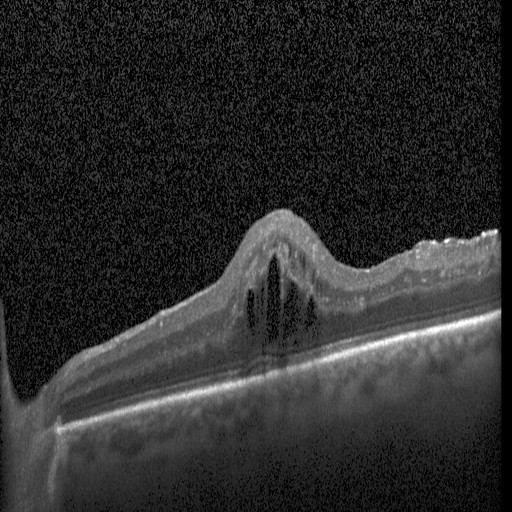
Spectral-domain OCT B-scan: DME.